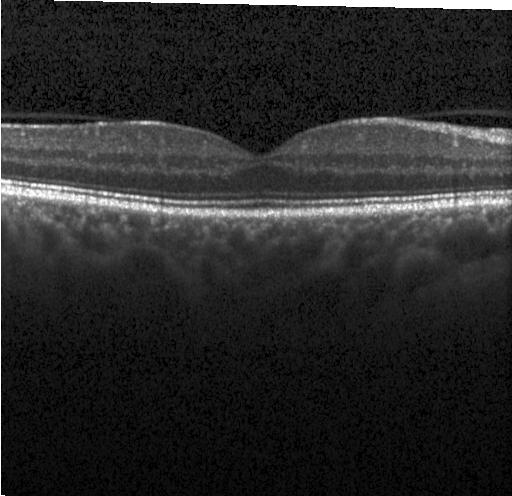
Retinal OCT cross-section; horizontal scan through the fovea; acquired on a Heidelberg Spectralis
Impression: no choroidal neovascularization, diabetic macular edema, or drusen.